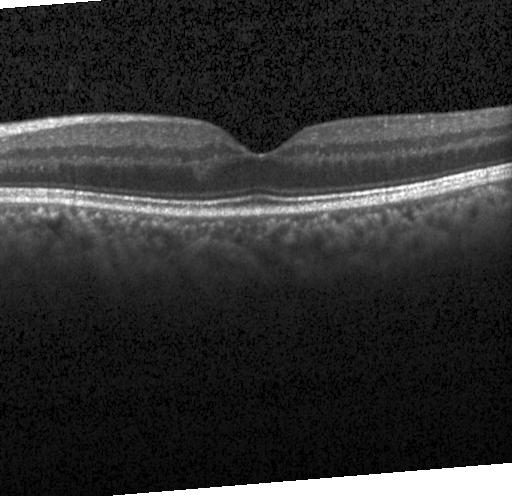 Optical coherence tomography scan — Assessment: no evidence of choroidal neovascularization, diabetic macular edema, or drusen.